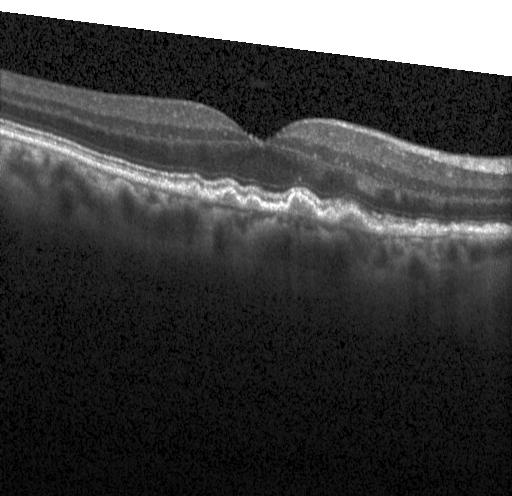

Dx: drusen.